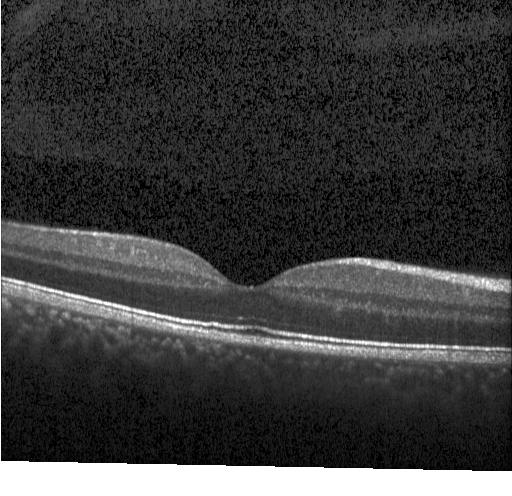
This B-scan demonstrates neither CNV, DME, nor drusen.